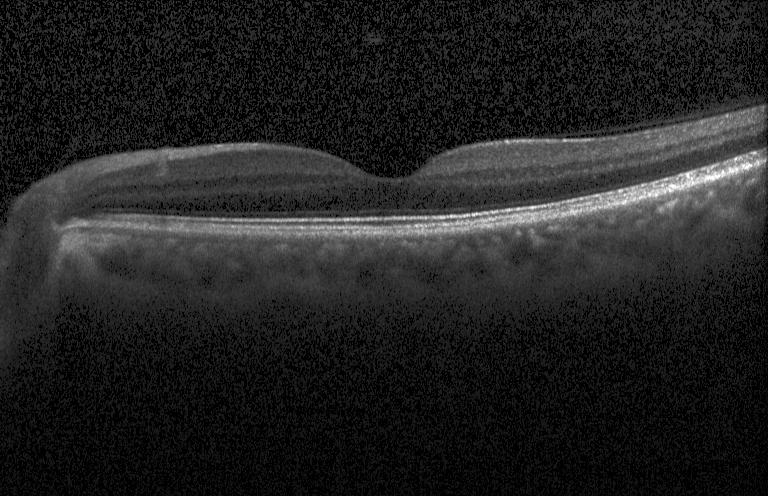

Retinal OCT B-scan. Centered on the fovea — No evidence of choroidal neovascularization, diabetic macular edema, or drusen.